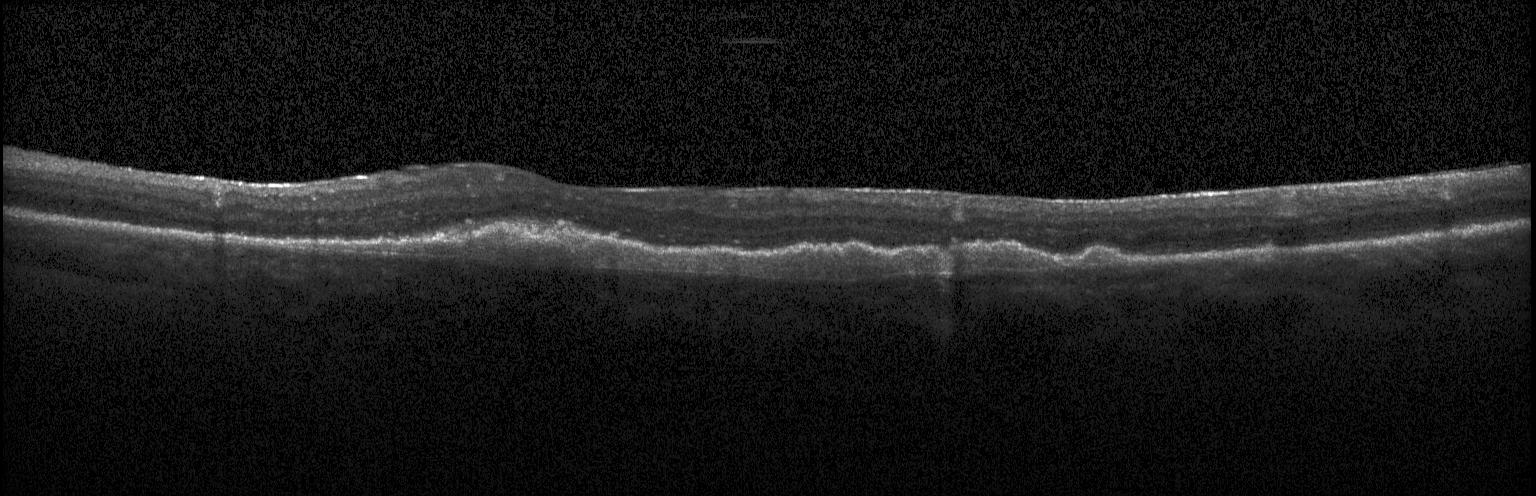 Heidelberg Spectralis; spectral-domain optical coherence tomography; optical coherence tomography scan. Dx: CNV.